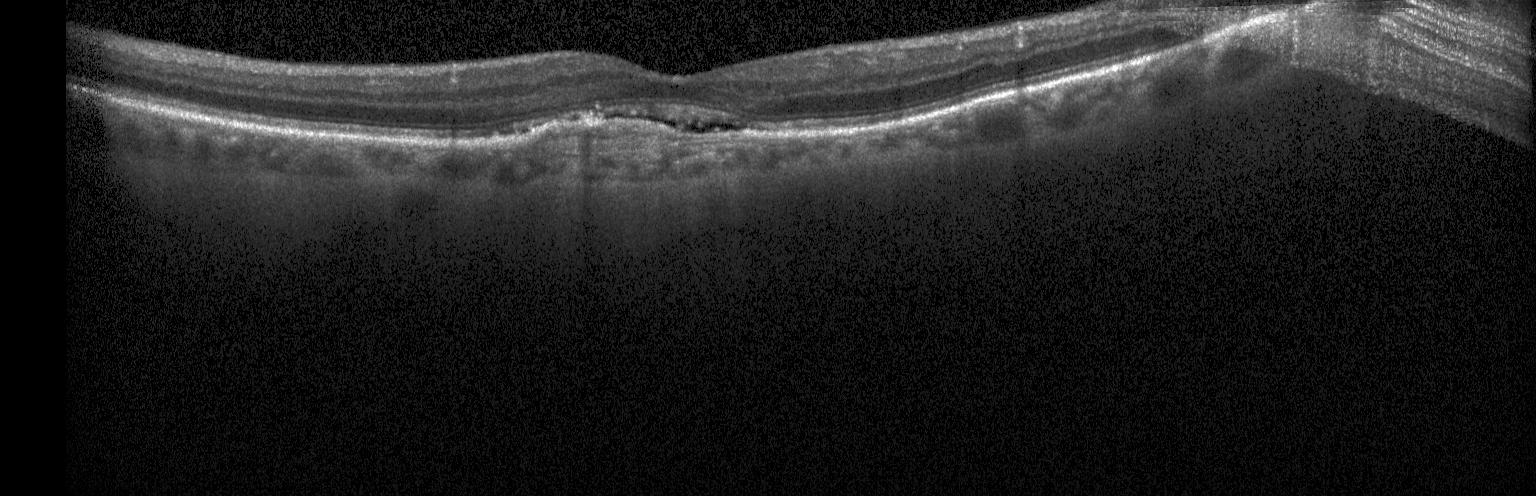 Spectral-domain optical coherence tomography, horizontal scan through the fovea, retinal OCT cross-section, acquired on a Heidelberg Spectralis. Diagnosis: a choroidal neovascular membrane.